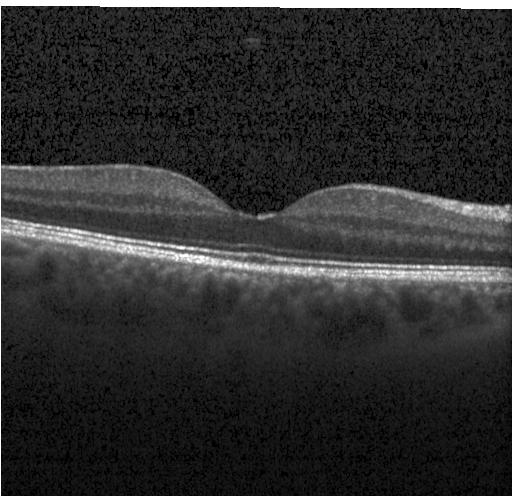 Retinal OCT cross-section showing neither choroidal neovascularization, diabetic macular edema, nor drusen.